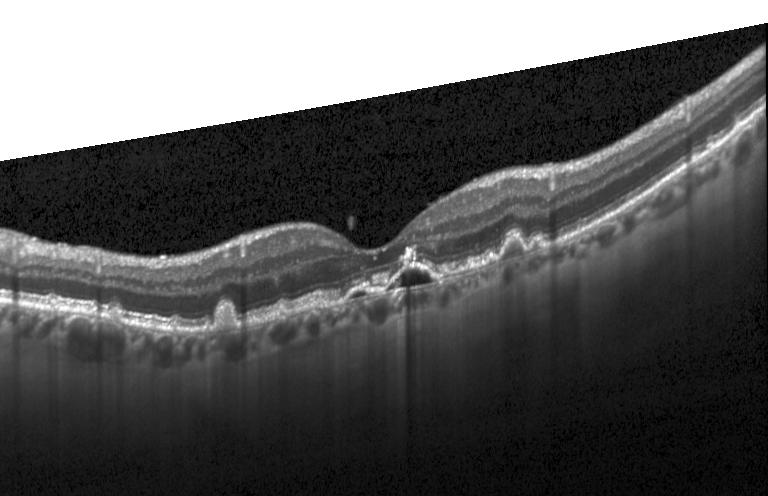 Optical coherence tomography B-scan.
Impression: a choroidal neovascular membrane.